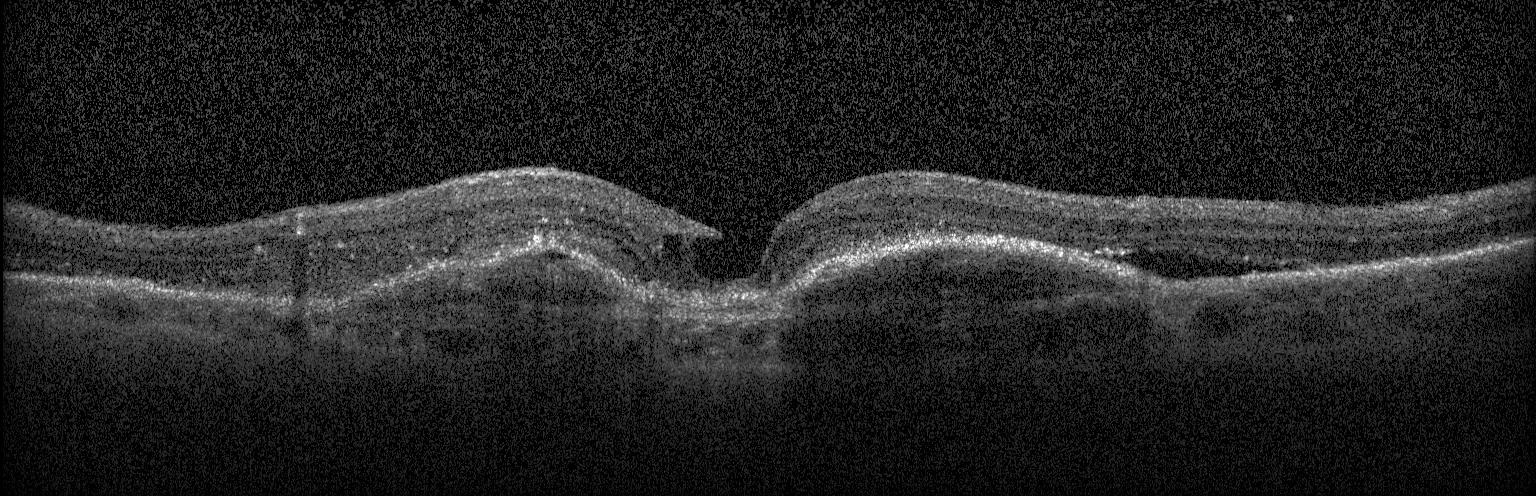

Retinal OCT cross-section. Choroidal neovascularization (CNV).